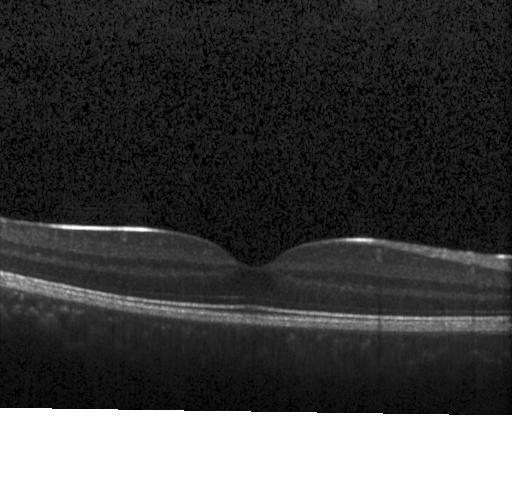 Instrument: Heidelberg Spectralis, centered on the fovea, spectral-domain OCT, retinal OCT B-scan
Impression: neither choroidal neovascularization, diabetic macular edema, nor drusen.